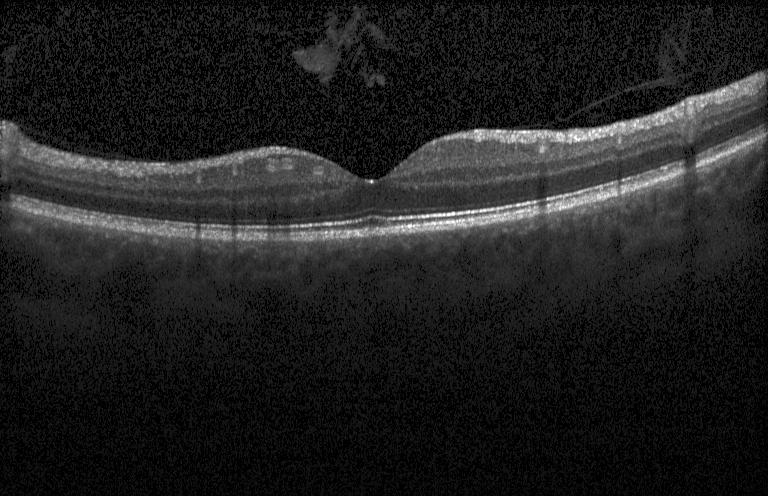

Diagnosis: no evidence of choroidal neovascularization, diabetic macular edema, or drusen.